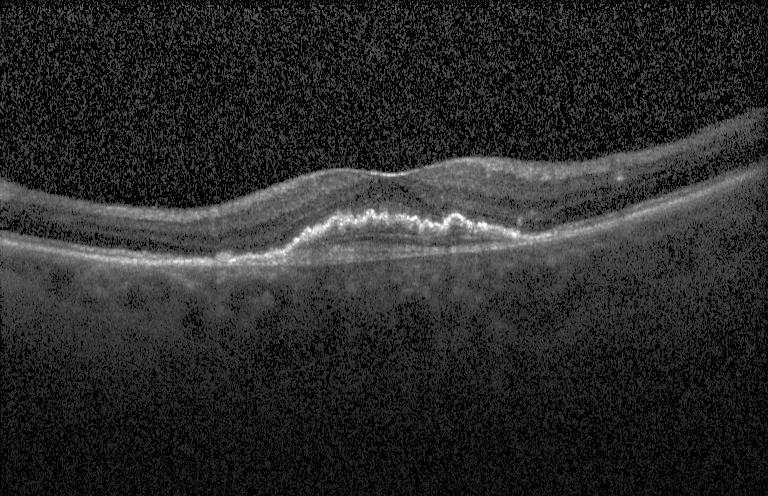

Instrument: Heidelberg Spectralis; optical coherence tomography scan; centered on the fovea.
The scan shows a choroidal neovascular membrane.